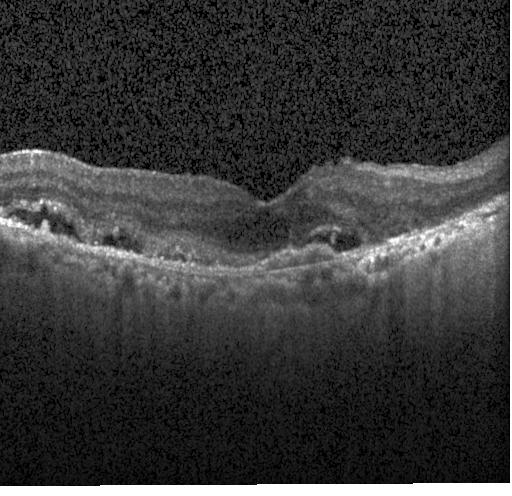

Optical coherence tomography scan. Finding: a choroidal neovascular membrane.